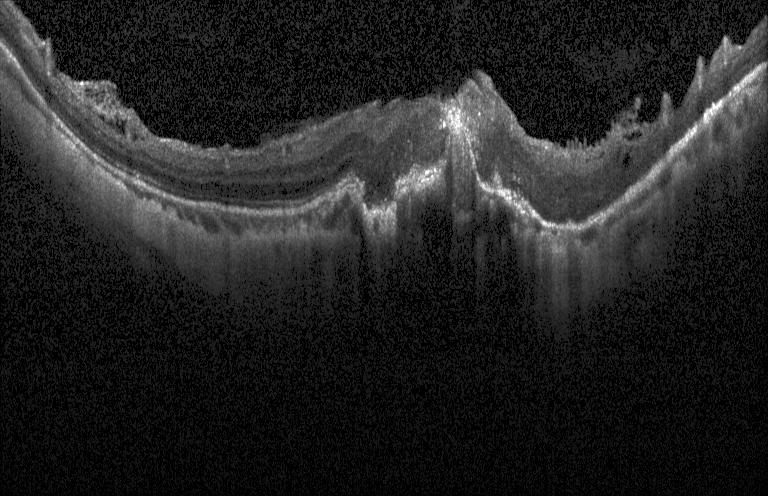
Spectral-domain OCT; retinal OCT cross-section; macular scan — This B-scan demonstrates choroidal neovascularization (CNV).